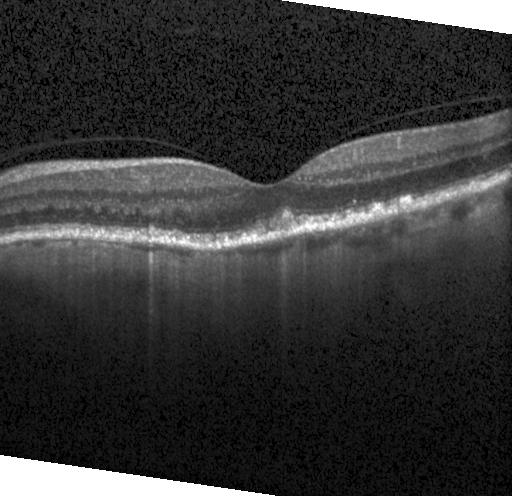 Diagnosis: multiple drusen.